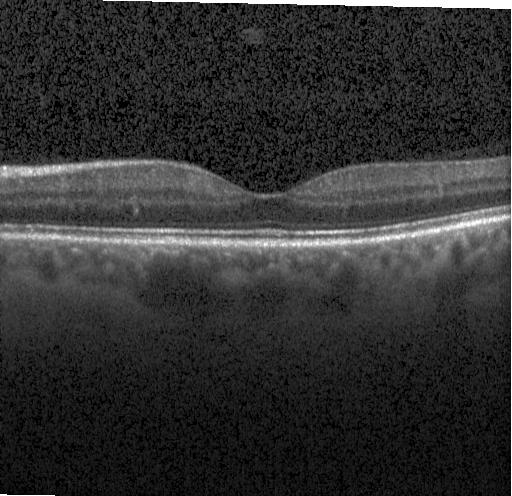
Heidelberg Spectralis OCT system. SD-OCT. Optical coherence tomography B-scan. Macular scan. Diagnosis: neither CNV, DME, nor drusen.